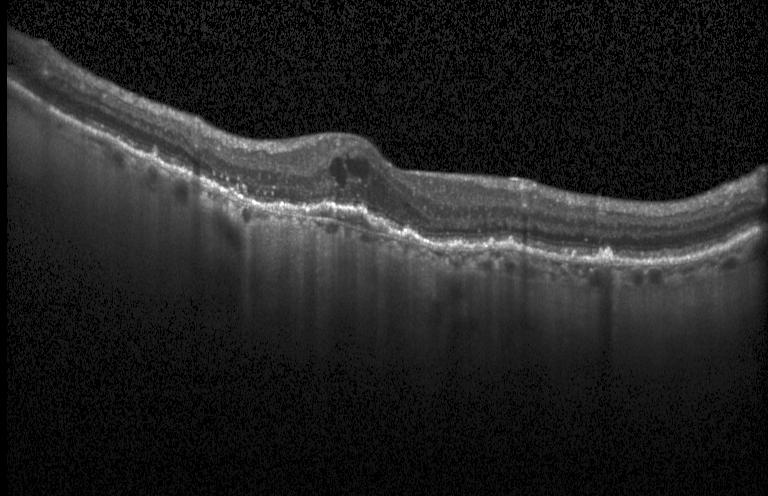 Optical coherence tomography scan, Heidelberg Spectralis. This B-scan demonstrates choroidal neovascularization.